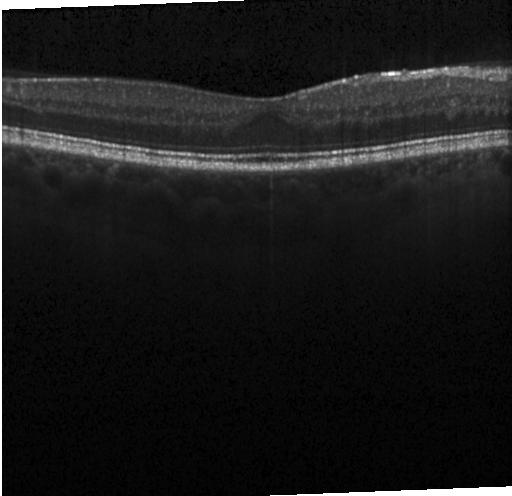

Retinal OCT cross-section showing neither CNV, DME, nor drusen.